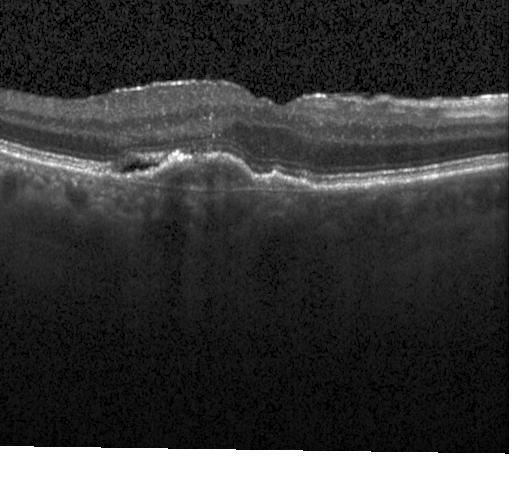 Spectral-domain optical coherence tomography · instrument: Heidelberg Spectralis · OCT line scan · centered on the fovea. Impression: choroidal neovascularization (CNV).